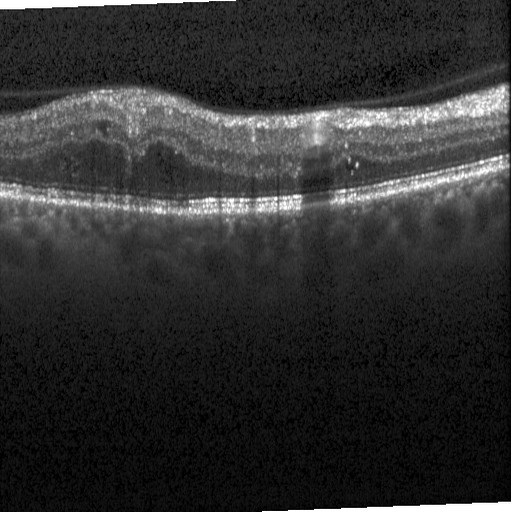
Impression: DME.